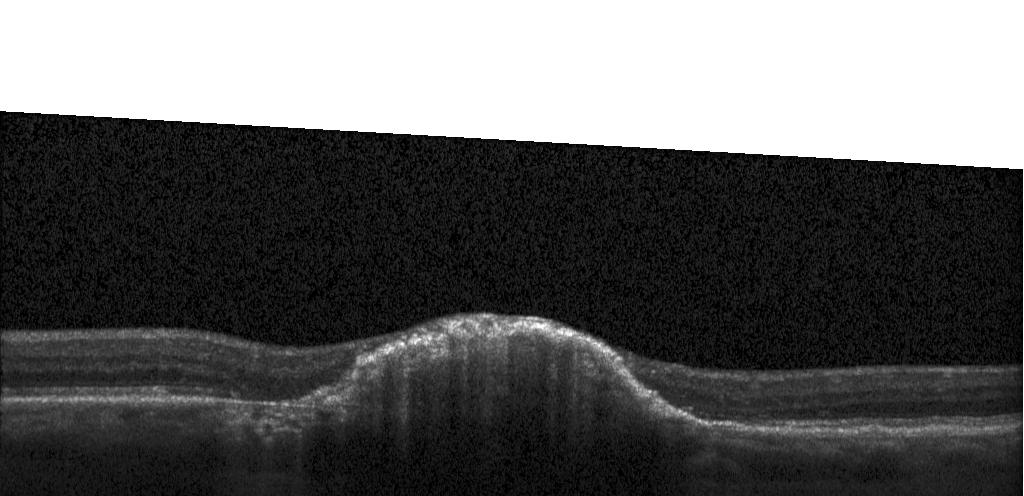

Optical coherence tomography scan. Macular scan
Finding: CNV.